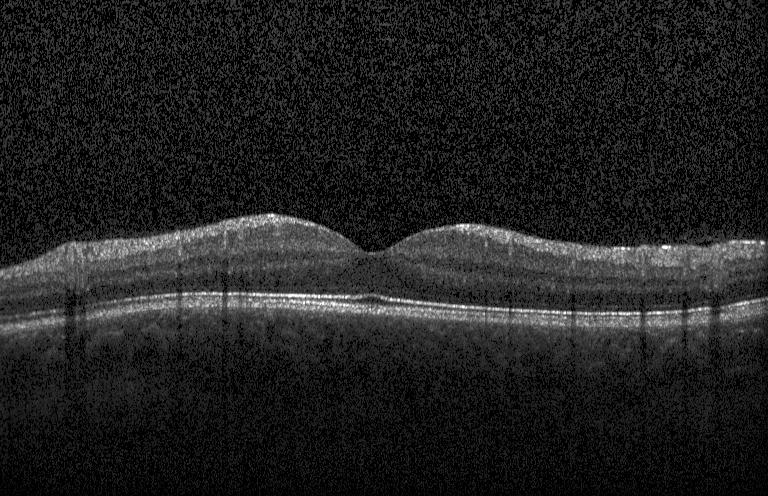

Optical coherence tomography B-scan. Fovea-centered. Heidelberg Spectralis. SD-OCT.
Impression: no evidence of choroidal neovascularization, diabetic macular edema, or drusen.